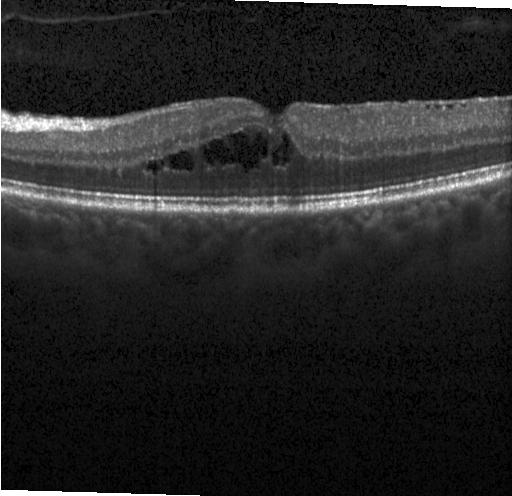

Centered on the fovea; OCT B-scan
Finding: diabetic macular edema (DME).